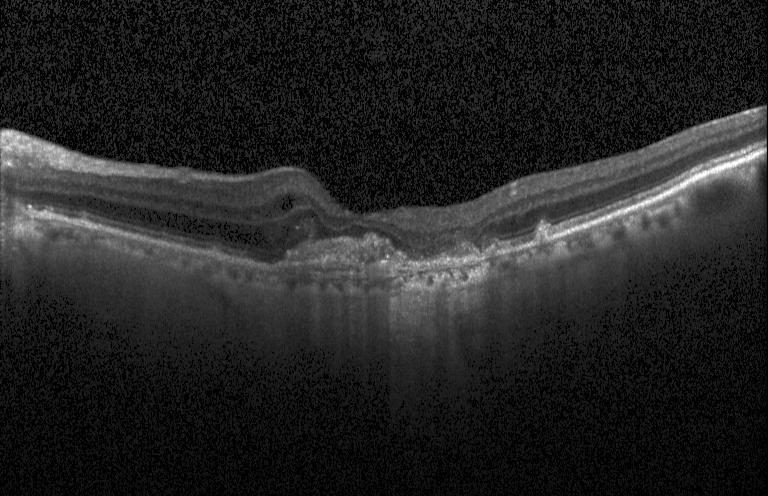 Retinal OCT cross-section
OCT finding: a choroidal neovascular membrane.